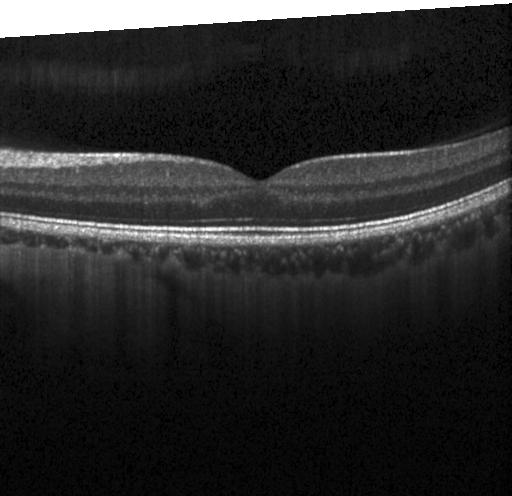 Optical coherence tomography scan.
Finding: no choroidal neovascularization, no diabetic macular edema, and no drusen.